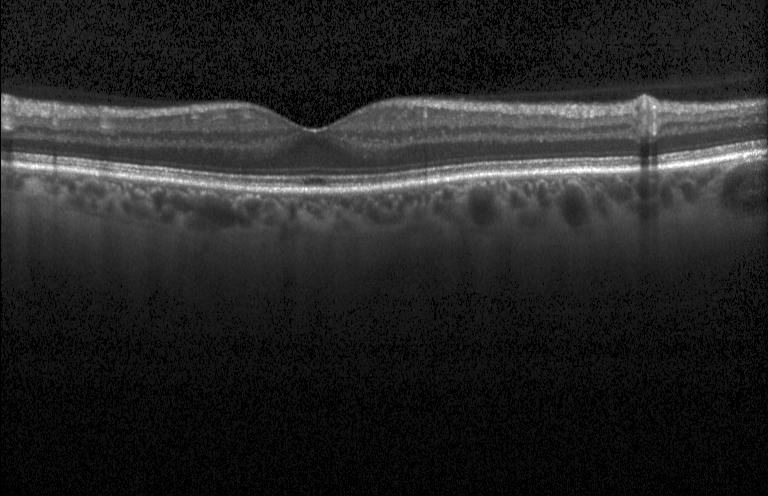 Optical coherence tomography B-scan. SD-OCT — No evidence of CNV, DME, or drusen.